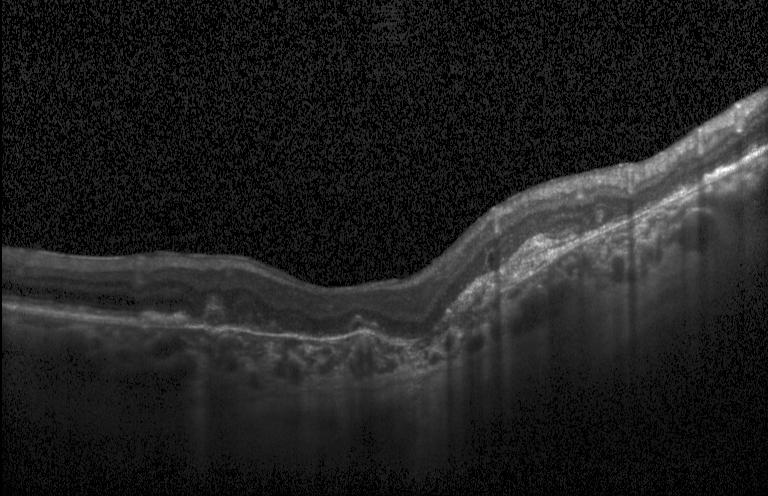

Finding: choroidal neovascularization (CNV).